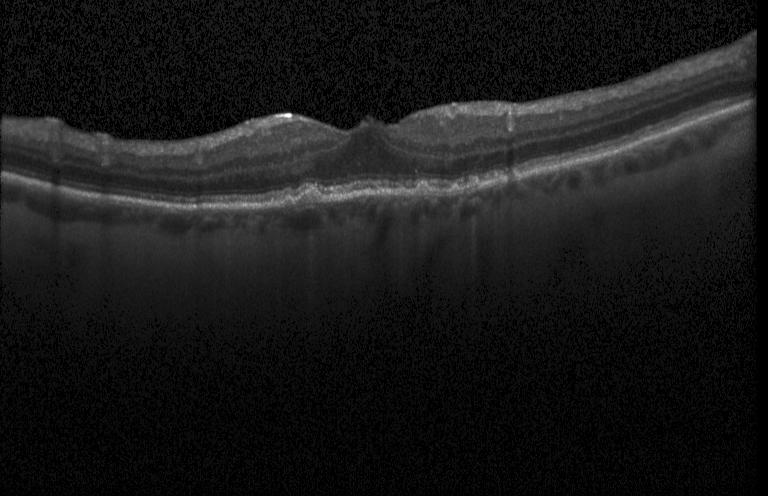
Heidelberg Spectralis · centered on the fovea · retinal OCT B-scan
Finding: multiple drusen.